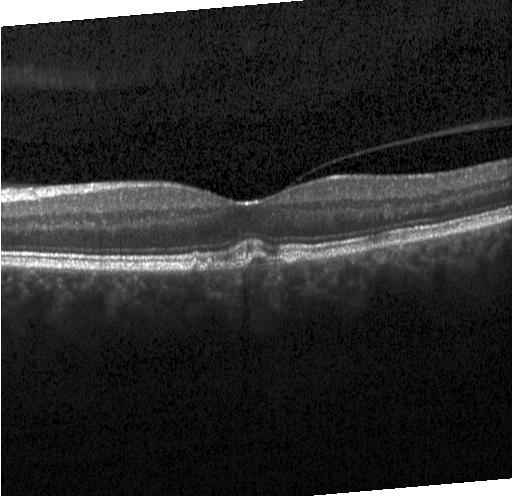
Macular OCT: drusen.